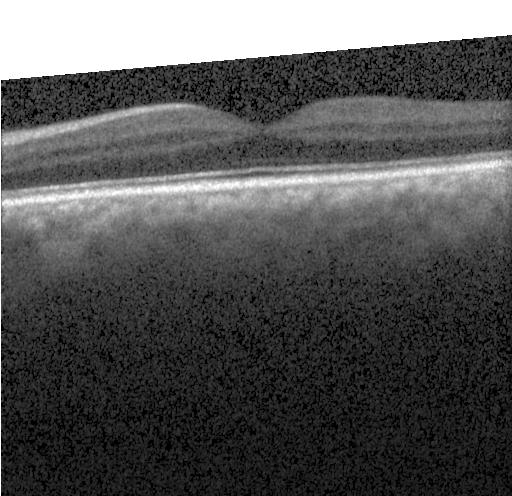

OCT line scan; Heidelberg Spectralis OCT system; centered on the fovea — Impression: no evidence of choroidal neovascularization, diabetic macular edema, or drusen.